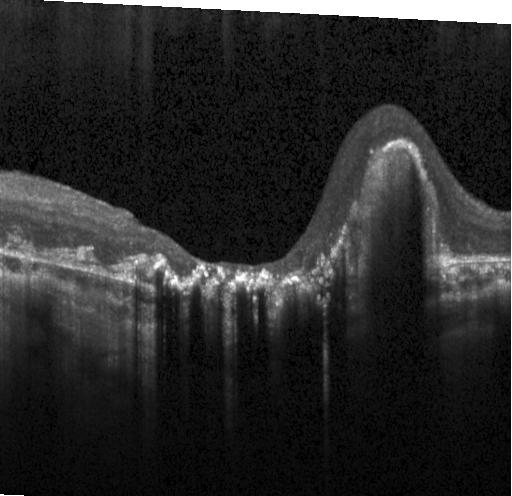
Macular scan · OCT line scan
Finding: choroidal neovascularization.